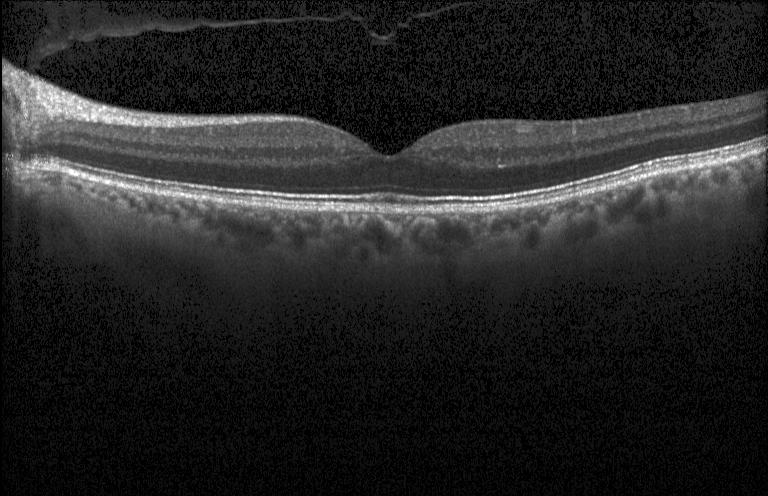

Through the macula, OCT B-scan — OCT finding: no evidence of choroidal neovascularization, diabetic macular edema, or drusen.